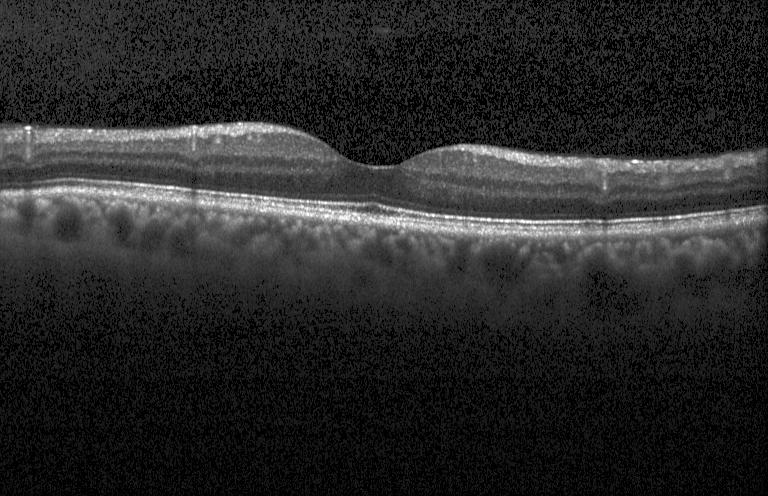

OCT line scan — No evidence of choroidal neovascularization, diabetic macular edema, or drusen.